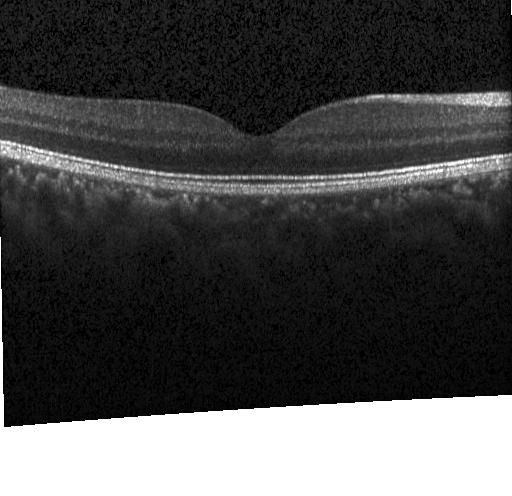

Optical coherence tomography B-scan · macular scan · spectral-domain optical coherence tomography
Diagnosis: no choroidal neovascularization, diabetic macular edema, or drusen.